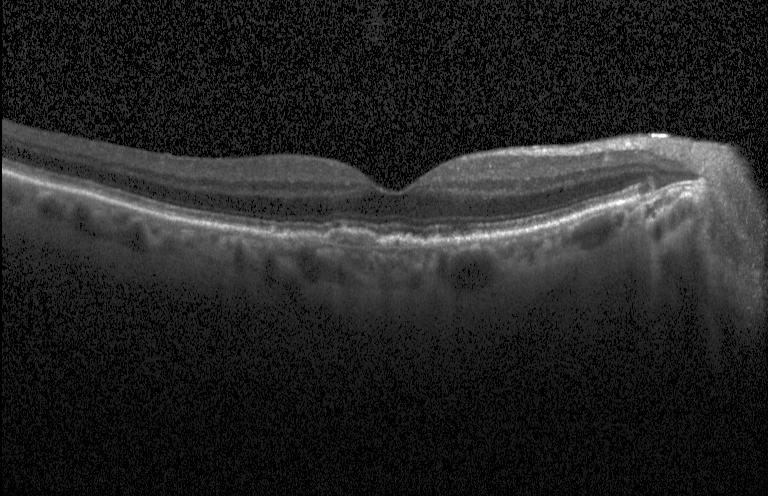 Finding: CNV.